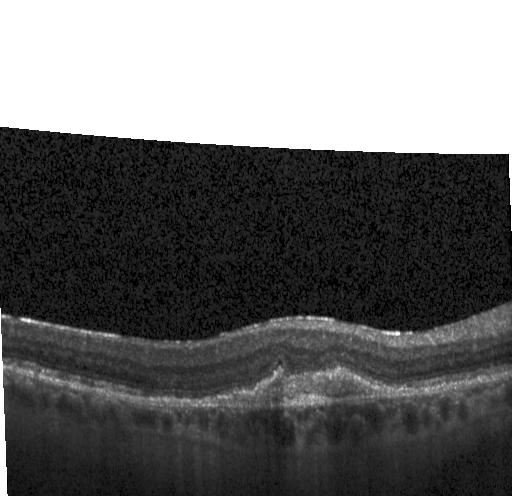
Macular OCT: choroidal neovascularization (CNV).